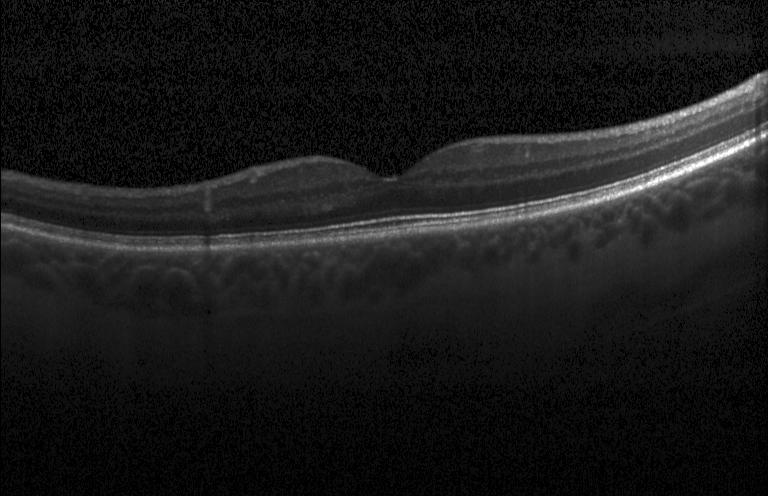

Neither CNV, DME, nor drusen.